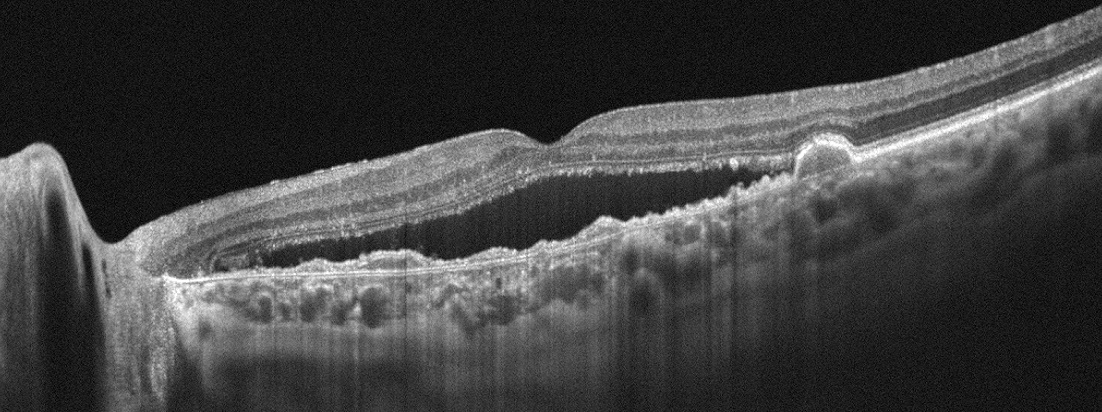 Retinal OCT cross-section. Instrument: Optovue Avanti RTVue XR. Finding: AMD.